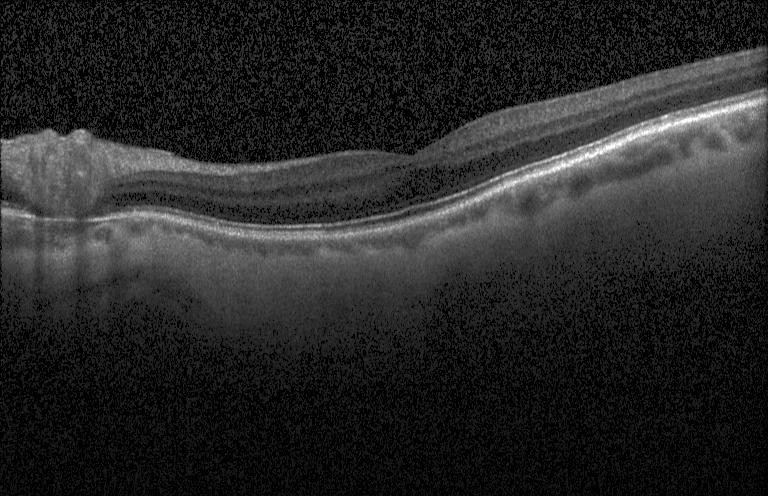
Spectral-domain OCT B-scan: no choroidal neovascularization, diabetic macular edema, or drusen.